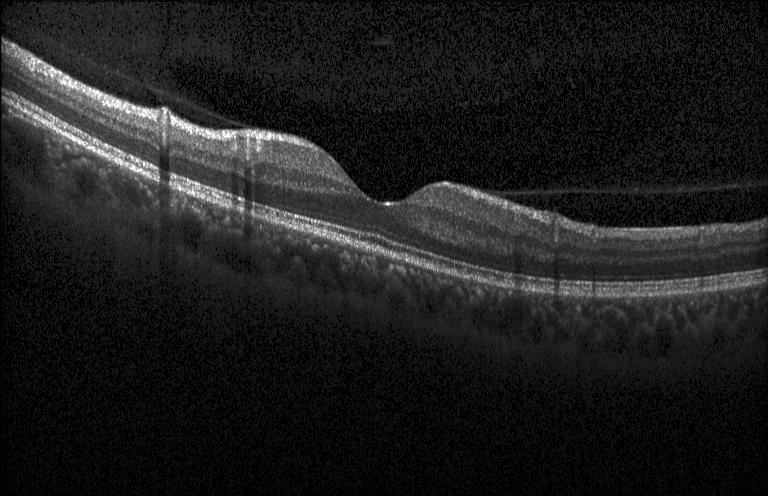
Spectral-domain optical coherence tomography, optical coherence tomography B-scan — This B-scan demonstrates no CNV, no DME, and no drusen.